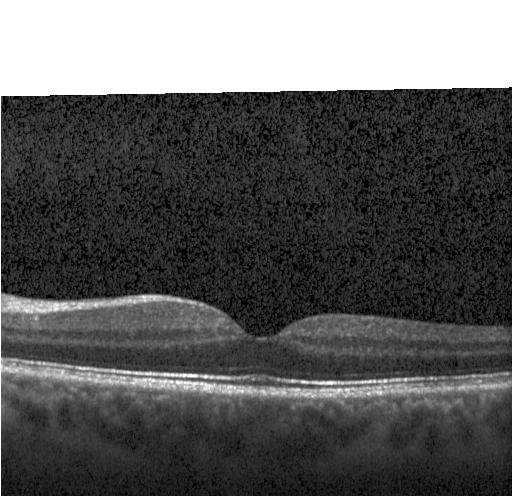
Heidelberg Spectralis OCT system · retinal OCT cross-section
Impression: neither CNV, DME, nor drusen.